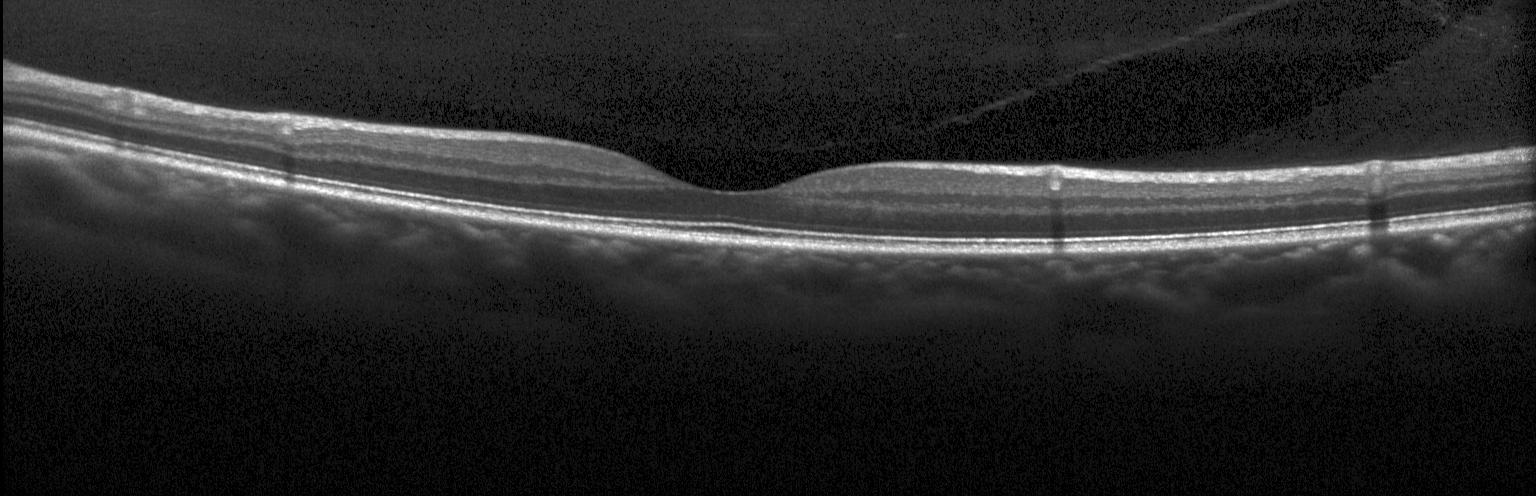 No choroidal neovascularization, diabetic macular edema, or drusen.